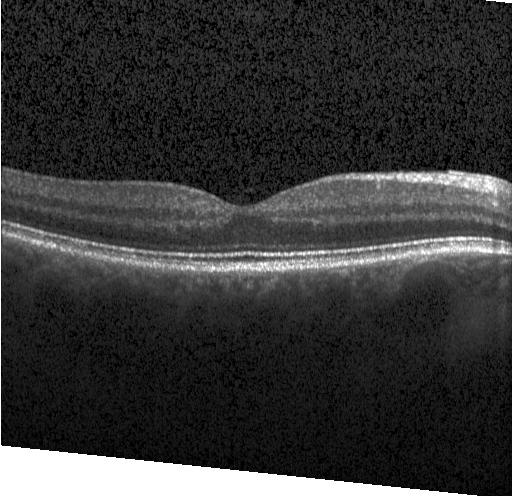 Heidelberg Spectralis; optical coherence tomography scan. Finding: no CNV, no DME, and no drusen.